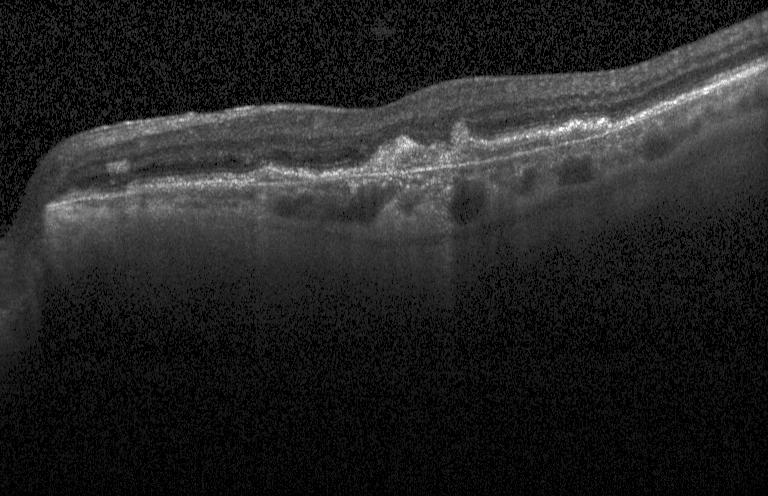
OCT line scan — Dx: a choroidal neovascular membrane.